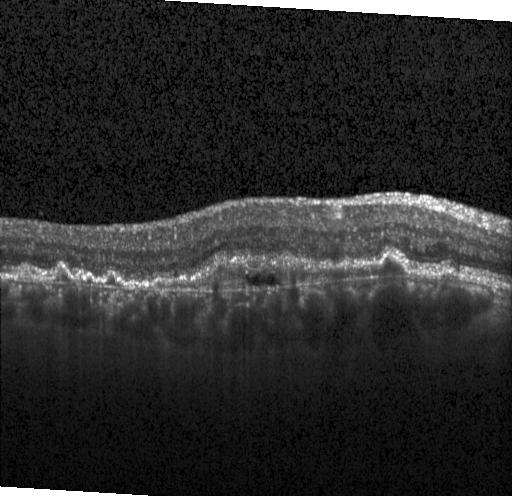
Fovea-centered; spectral-domain OCT; retinal OCT cross-section; acquired on a Heidelberg Spectralis — OCT finding: a choroidal neovascular membrane.